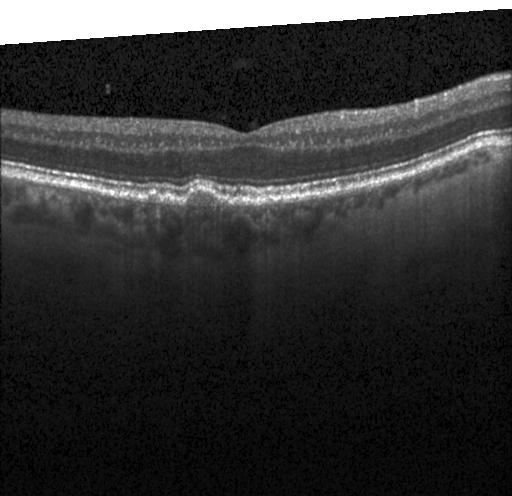

This B-scan demonstrates multiple drusen.